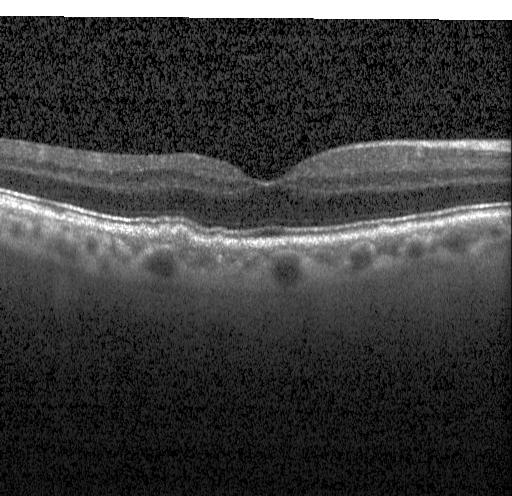

Retinal OCT cross-section · macular scan · spectral-domain optical coherence tomography. Macular OCT: drusen.